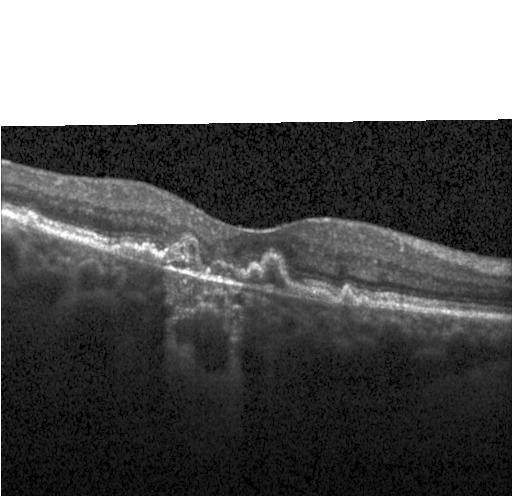
The scan shows CNV.